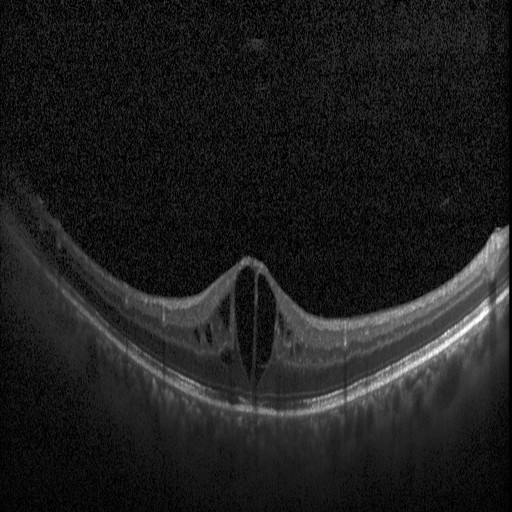 The scan shows DME.